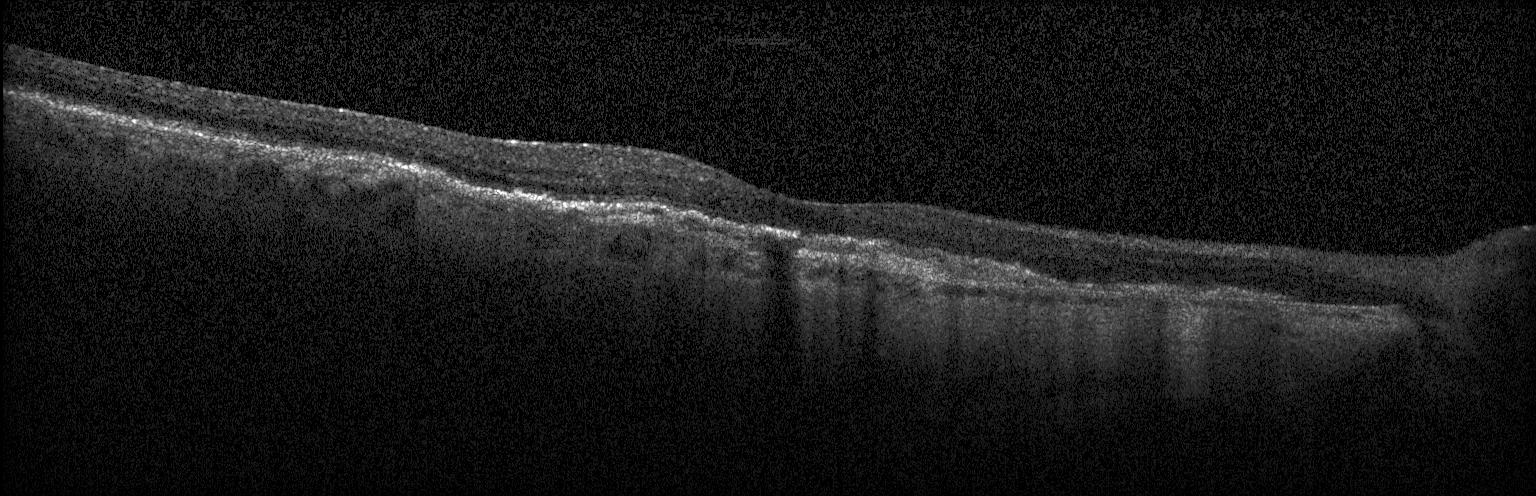

Retinal OCT B-scan.
Impression: a choroidal neovascular membrane.